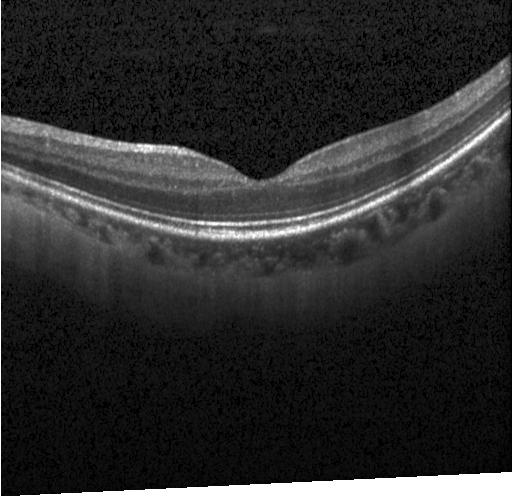

Retinal OCT B-scan — OCT finding: no evidence of choroidal neovascularization, diabetic macular edema, or drusen.